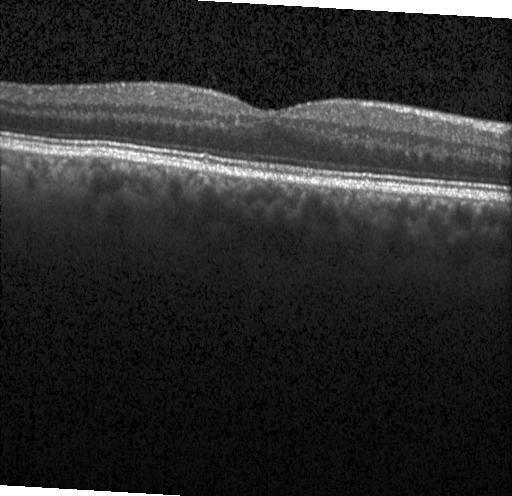 Centered on the fovea · acquired on a Heidelberg Spectralis · optical coherence tomography B-scan — Finding: no CNV, no DME, and no drusen.